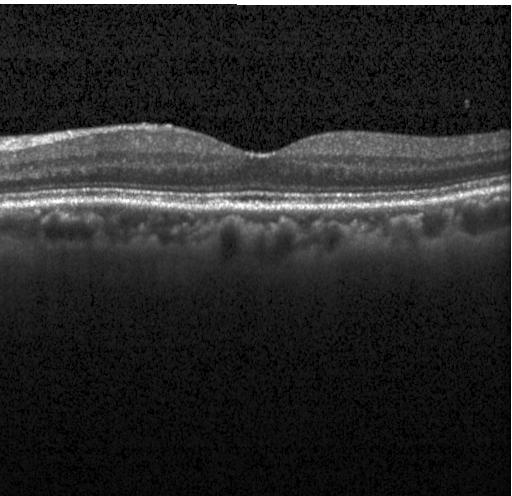 Retinal OCT cross-section.
Macular OCT: no choroidal neovascularization, diabetic macular edema, or drusen.